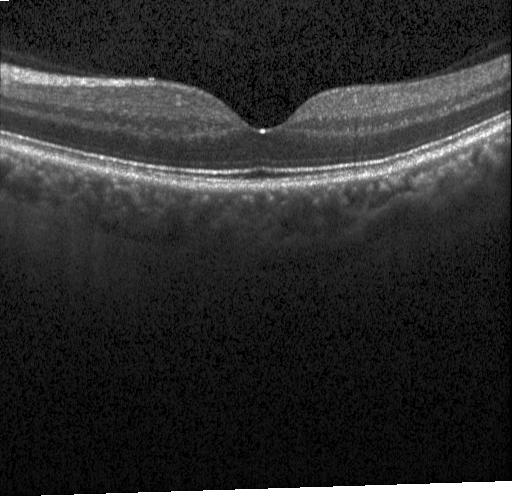

Optical coherence tomography B-scan, Heidelberg Spectralis OCT system, spectral-domain OCT. No evidence of choroidal neovascularization, diabetic macular edema, or drusen.